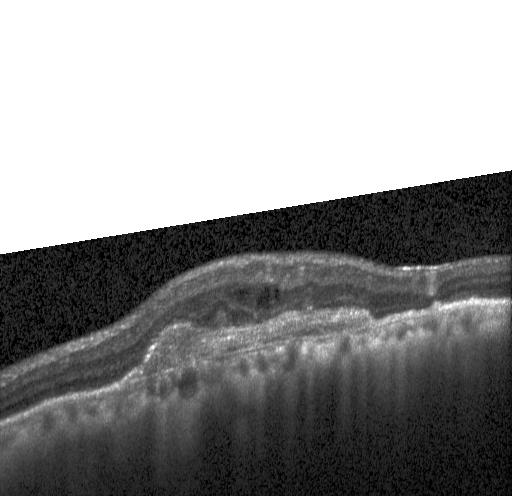

This B-scan demonstrates choroidal neovascularization (CNV).